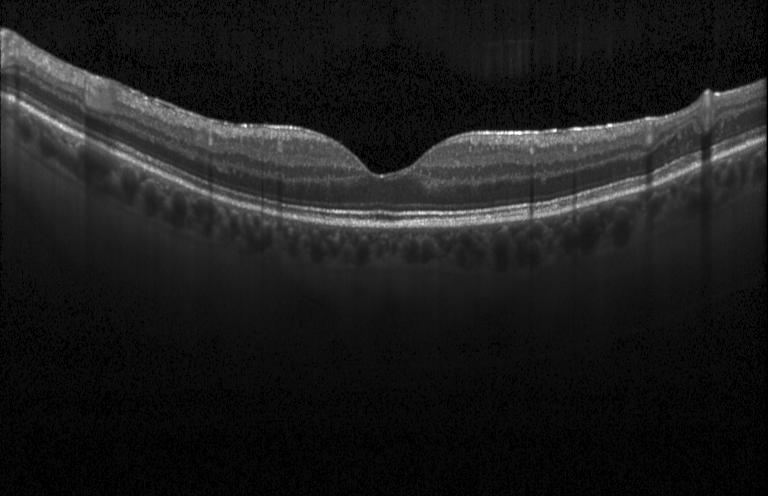

OCT finding: no CNV, no DME, and no drusen.